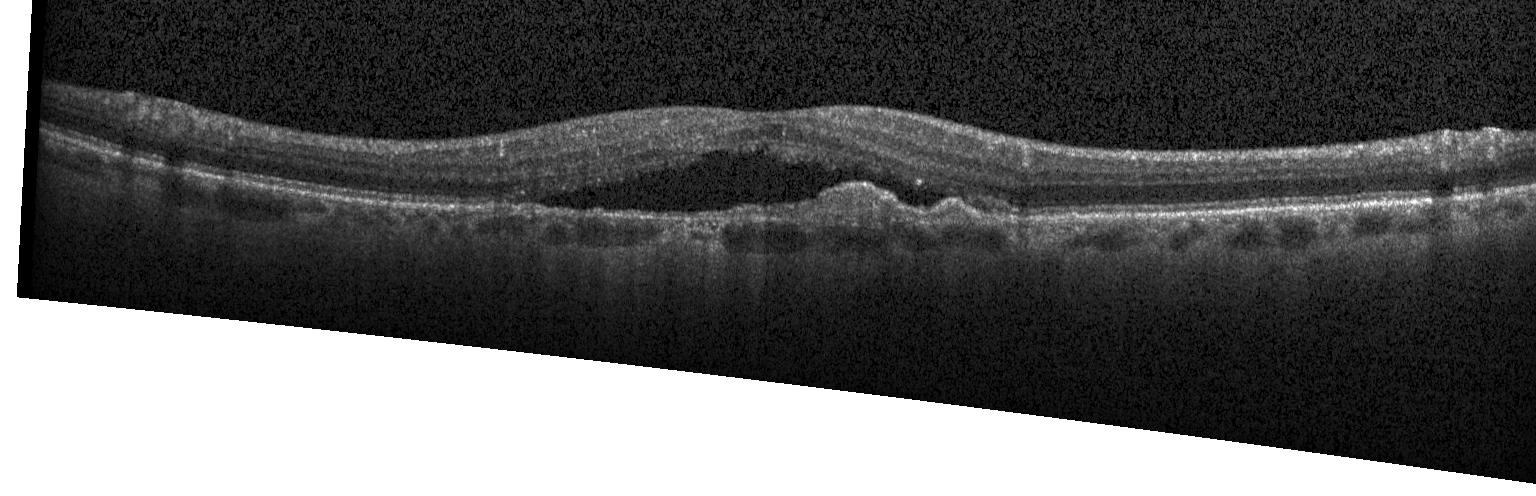 Instrument: Heidelberg Spectralis. Optical coherence tomography B-scan. SD-OCT. Macular scan — Diagnosis: choroidal neovascularization (CNV).